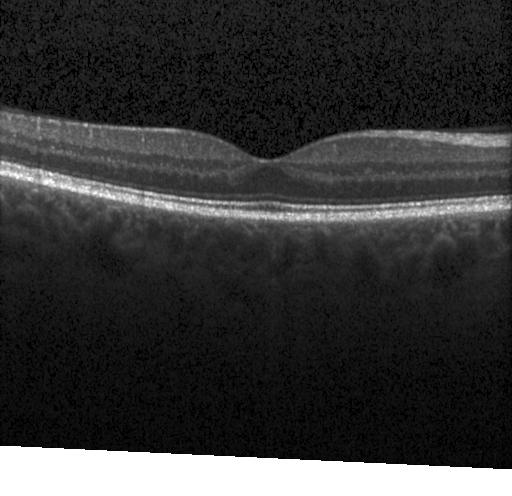

Impression: no CNV, no DME, and no drusen.